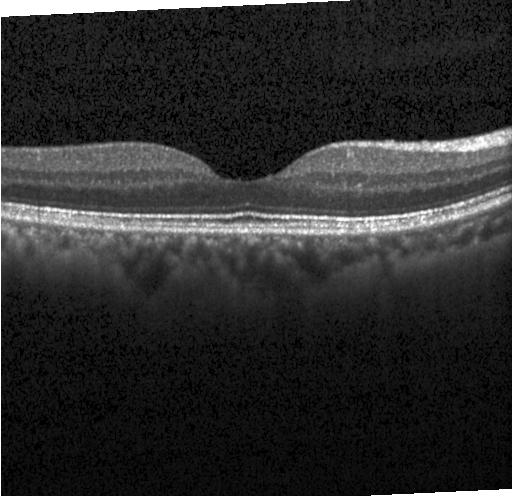 Spectral-domain OCT · through the macula · acquired on a Heidelberg Spectralis · optical coherence tomography scan
Diagnosis: no evidence of choroidal neovascularization, diabetic macular edema, or drusen.